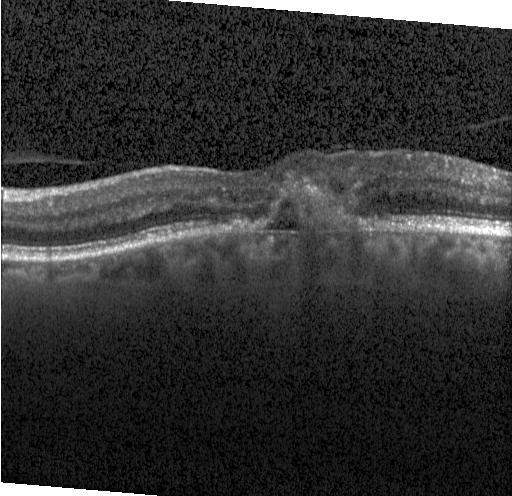
OCT B-scan — Dx: a choroidal neovascular membrane.